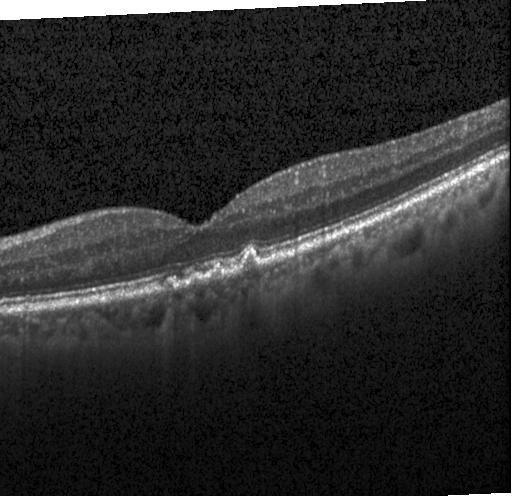
Fovea-centered, Heidelberg Spectralis OCT system, optical coherence tomography B-scan, spectral-domain optical coherence tomography.
Assessment: multiple drusen.